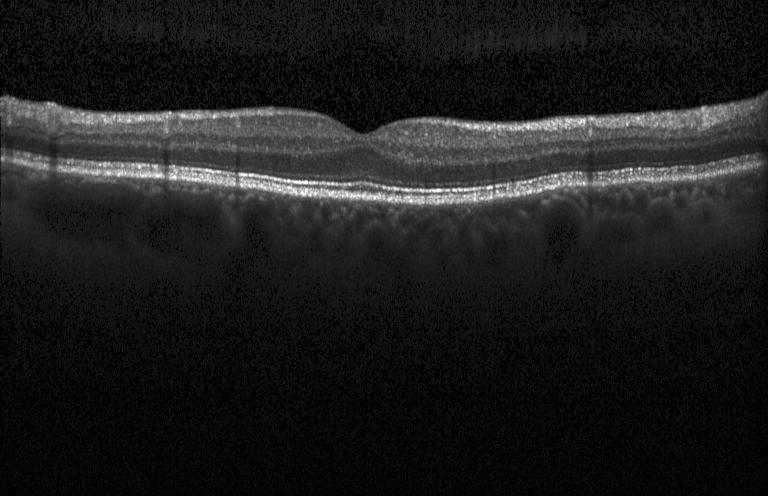
Retinal OCT cross-section; macular scan; Heidelberg Spectralis.
No CNV, no DME, and no drusen.